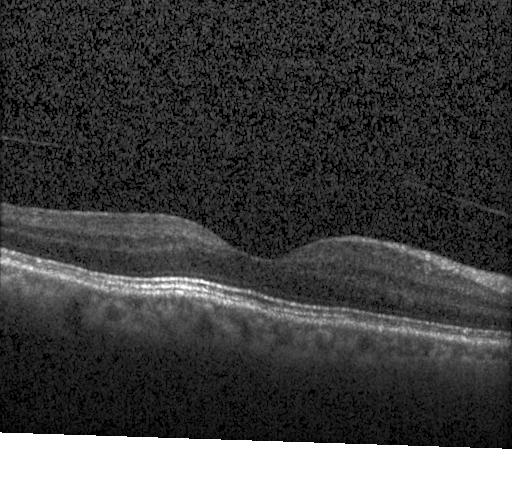
SD-OCT, OCT line scan, Heidelberg Spectralis. Assessment: no choroidal neovascularization, diabetic macular edema, or drusen.